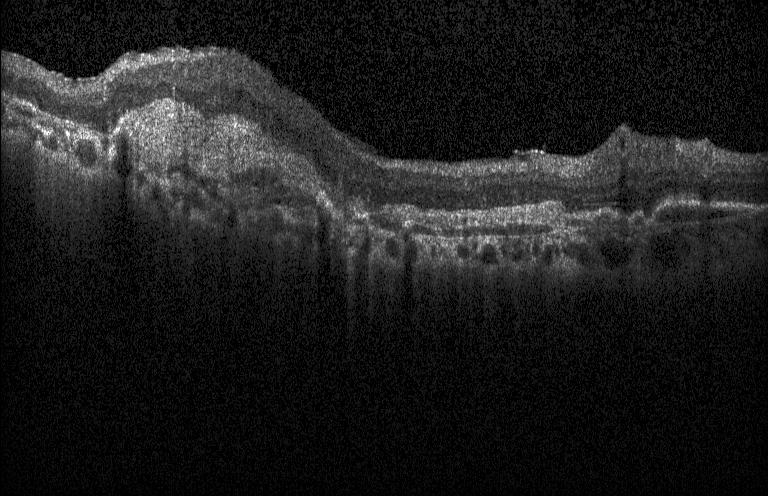 The scan shows a choroidal neovascular membrane.